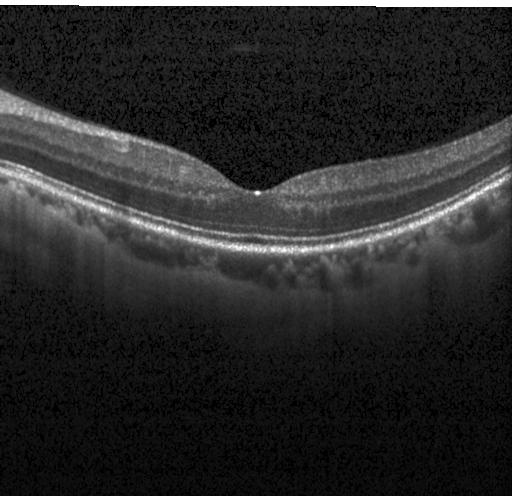

No choroidal neovascularization, no diabetic macular edema, and no drusen.